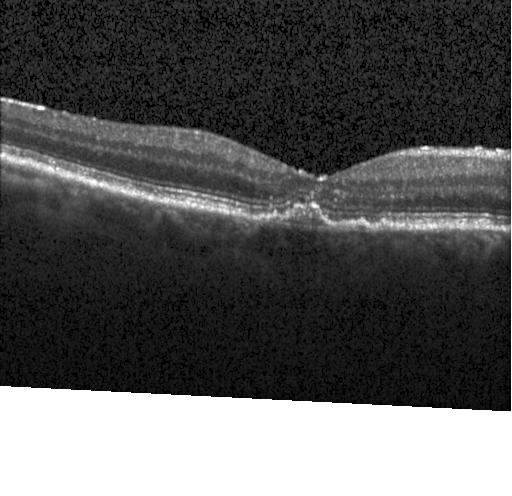 OCT scan showing sub-RPE drusenoid deposits.